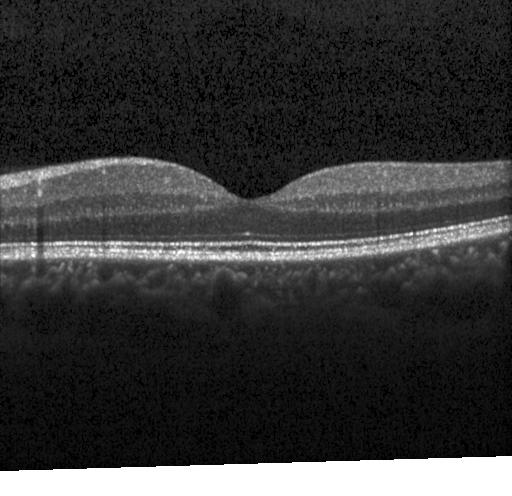

SD-OCT; optical coherence tomography B-scan.
The scan shows neither choroidal neovascularization, diabetic macular edema, nor drusen.